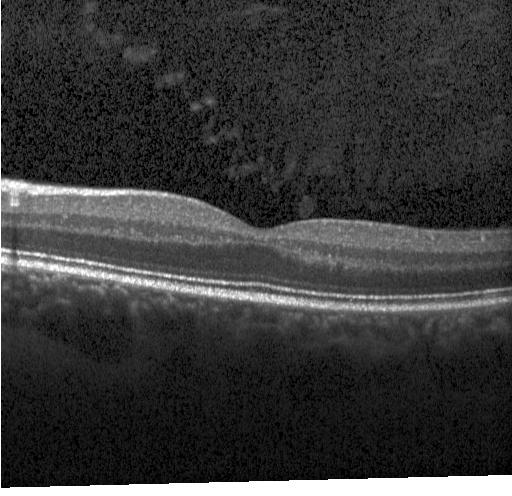

OCT finding: no choroidal neovascularization, no diabetic macular edema, and no drusen.